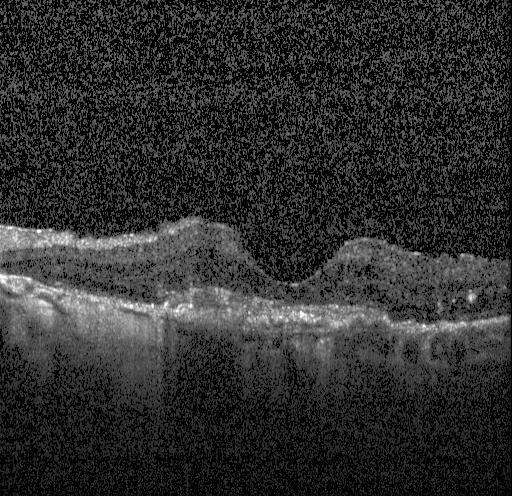 Macular OCT: choroidal neovascularization.